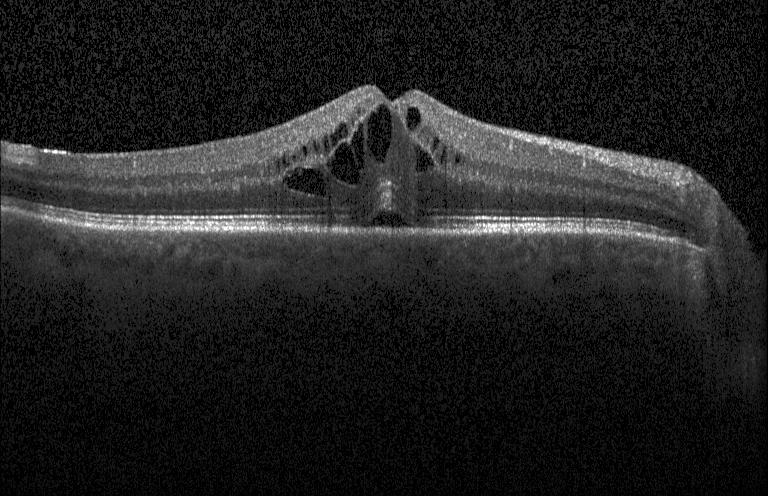

Diagnosis: diabetic macular edema (DME).